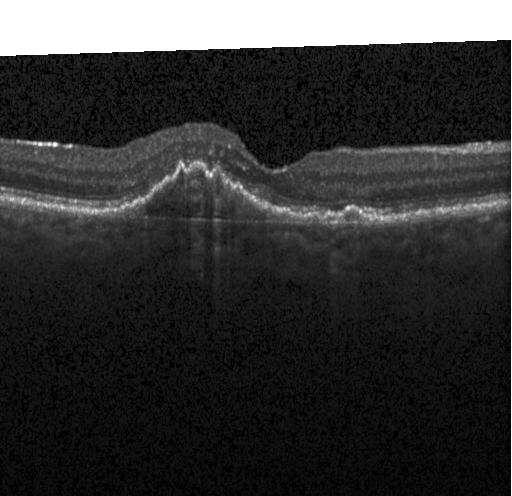
Impression: a choroidal neovascular membrane.